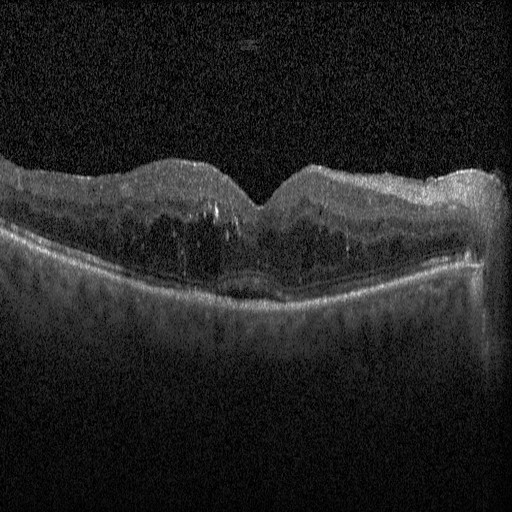 Heidelberg Spectralis OCT system; optical coherence tomography B-scan
This B-scan demonstrates DME.